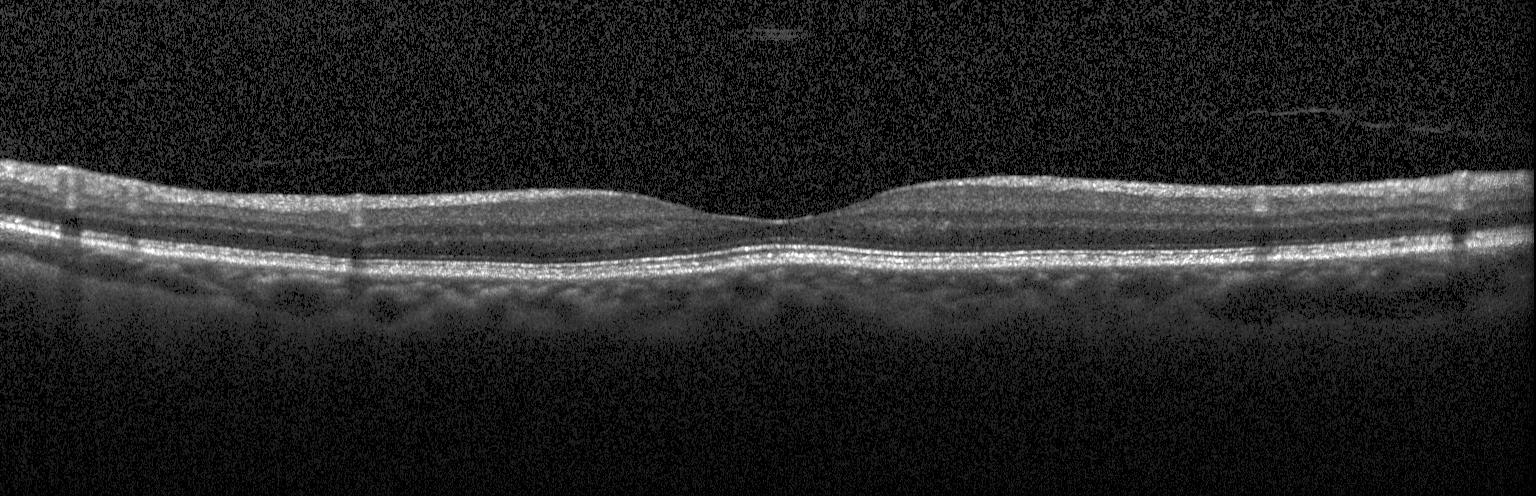

Retinal OCT cross-section.
This B-scan demonstrates no choroidal neovascularization, diabetic macular edema, or drusen.